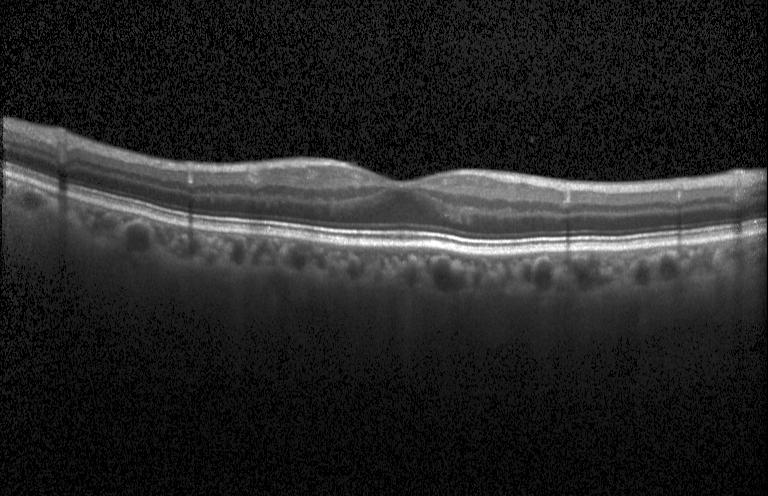 Diagnosis: no choroidal neovascularization, diabetic macular edema, or drusen.